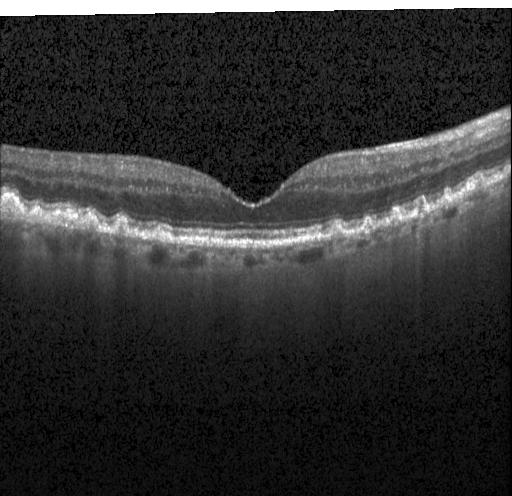

OCT B-scan; spectral-domain optical coherence tomography. The scan shows sub-RPE drusenoid deposits.